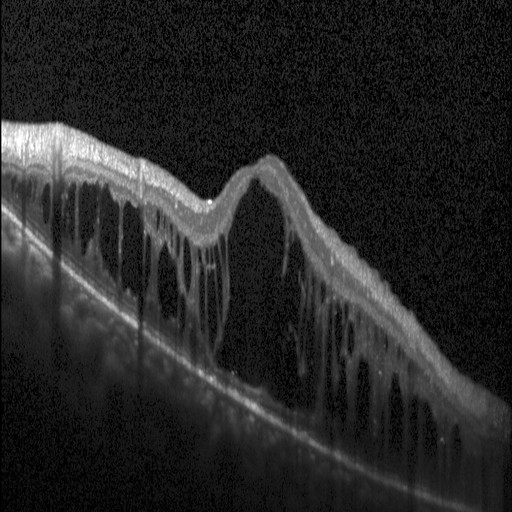 Spectral-domain OCT; optical coherence tomography B-scan.
Finding: diabetic macular edema.